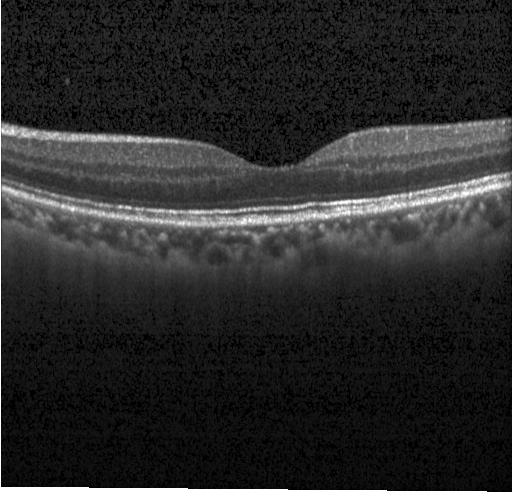

Optical coherence tomography scan. Heidelberg Spectralis. Spectral-domain OCT. Centered on the fovea
Assessment: neither choroidal neovascularization, diabetic macular edema, nor drusen.